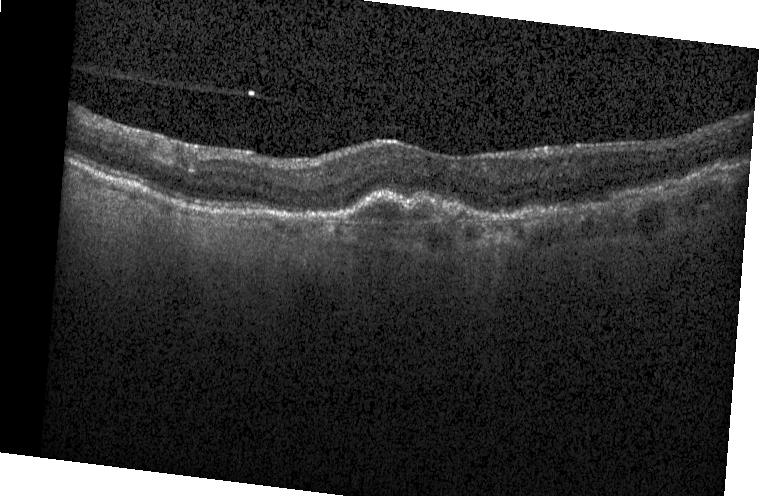 Retinal OCT cross-section. Macular scan. Spectral-domain OCT. Heidelberg Spectralis OCT system. Dx: CNV.